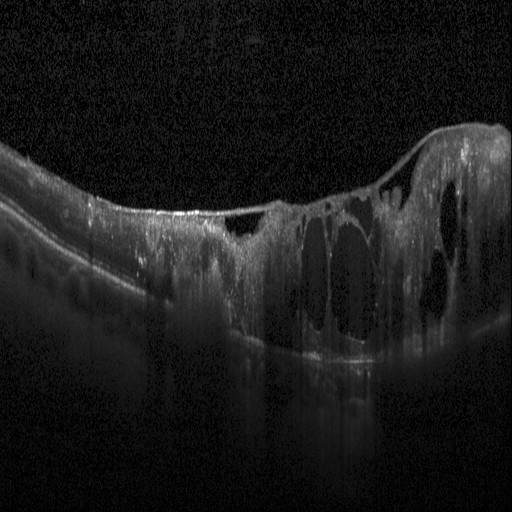
Macular OCT: diabetic macular edema.